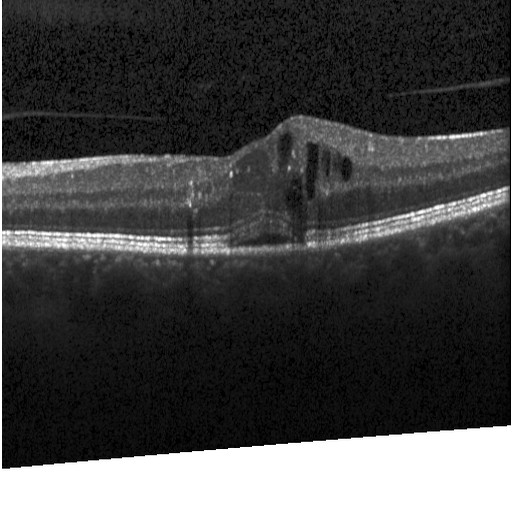
Diagnosis: diabetic macular edema (DME).